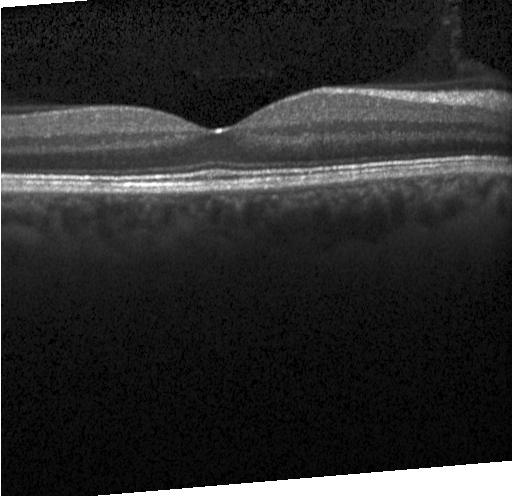
Macular scan, optical coherence tomography scan — No CNV, no DME, and no drusen.